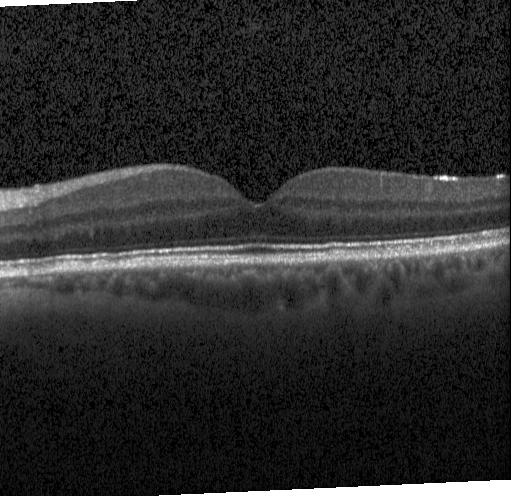

Retinal OCT cross-section, instrument: Heidelberg Spectralis, SD-OCT — Impression: neither choroidal neovascularization, diabetic macular edema, nor drusen.